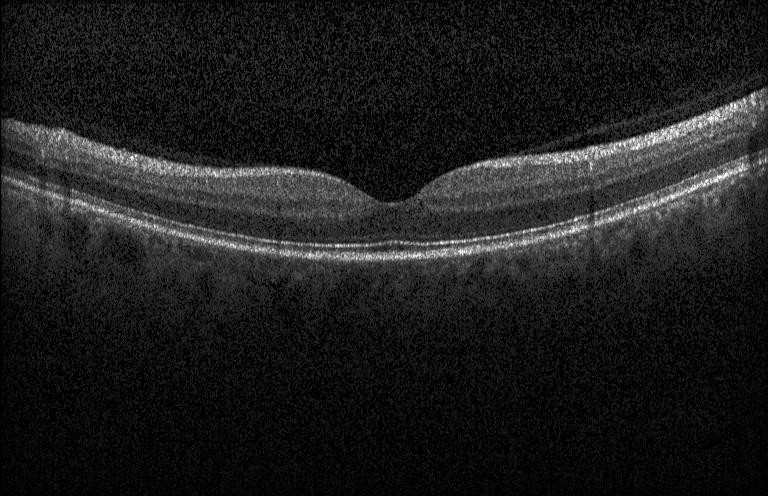

Heidelberg Spectralis, OCT B-scan, horizontal scan through the fovea
Dx: neither CNV, DME, nor drusen.